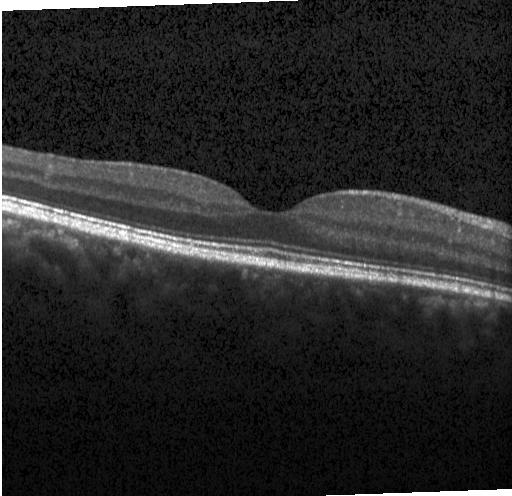
Heidelberg Spectralis. SD-OCT. Fovea-centered. OCT B-scan — Finding: no choroidal neovascularization, diabetic macular edema, or drusen.